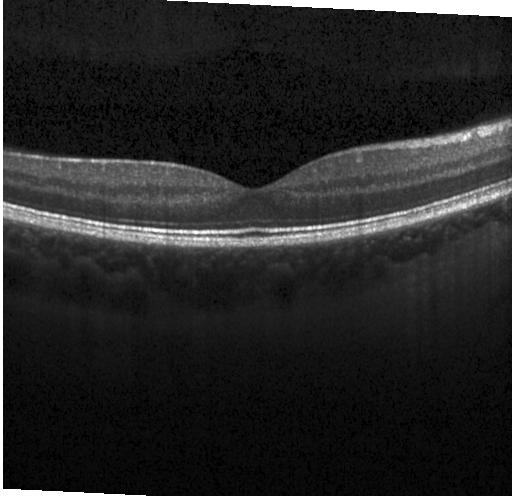
Macular OCT: neither CNV, DME, nor drusen.